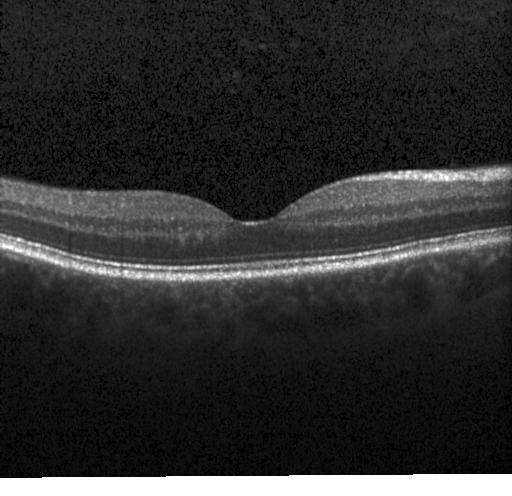 Fovea-centered, spectral-domain optical coherence tomography, acquired on a Heidelberg Spectralis, OCT line scan.
Diagnosis: no evidence of choroidal neovascularization, diabetic macular edema, or drusen.